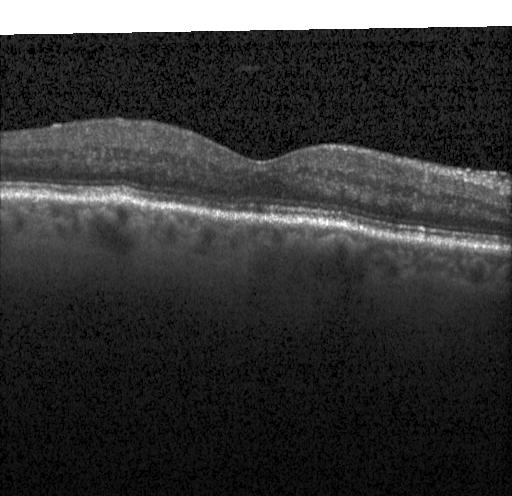
Impression: no CNV, DME, or drusen.